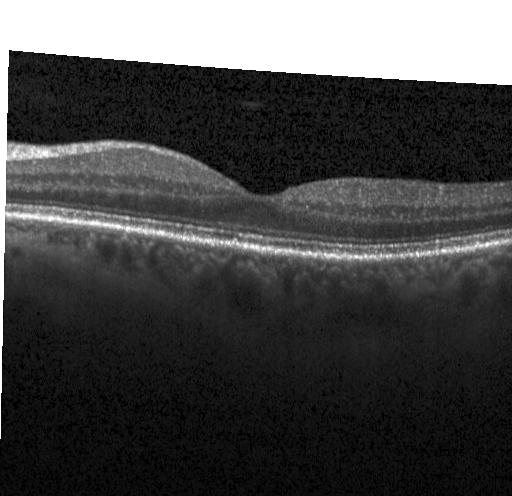 Heidelberg Spectralis OCT system. Optical coherence tomography B-scan. Spectral-domain optical coherence tomography — OCT finding: neither choroidal neovascularization, diabetic macular edema, nor drusen.